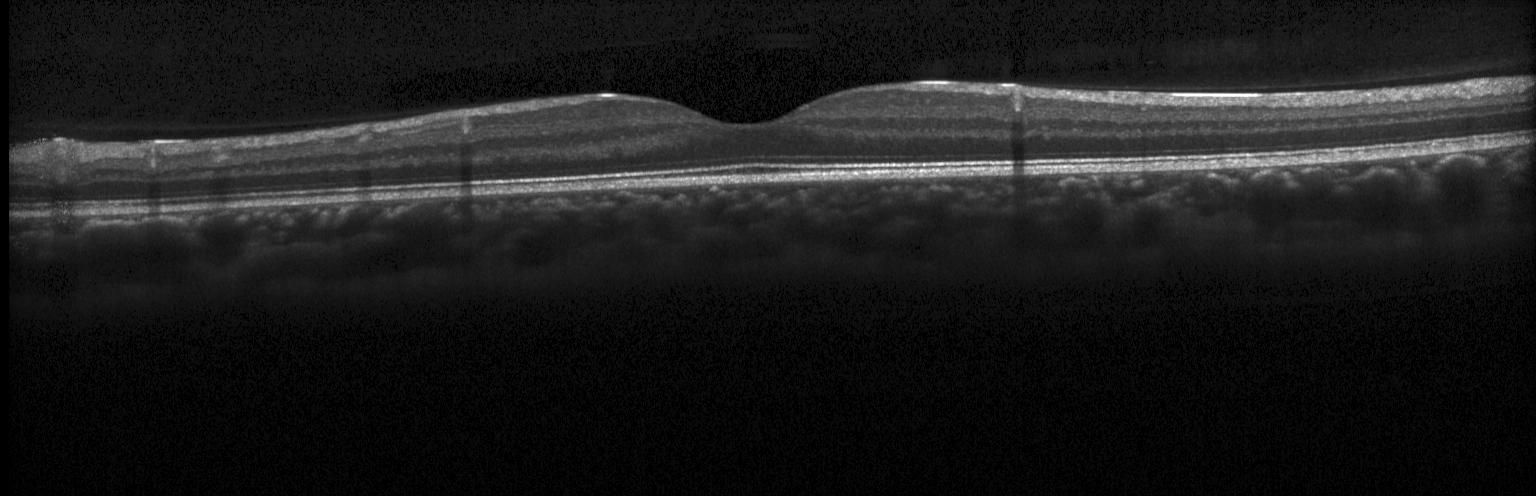
OCT B-scan
Diagnosis: no evidence of choroidal neovascularization, diabetic macular edema, or drusen.